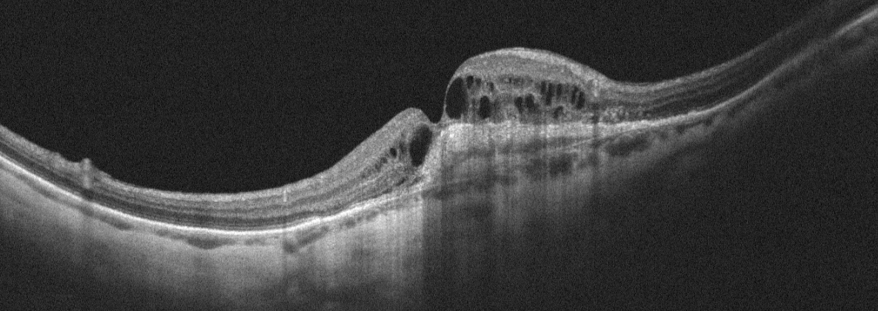

Through the macula · Optovue Avanti RTVue XR · optical coherence tomography B-scan.
Impression: age-related macular degeneration (AMD).